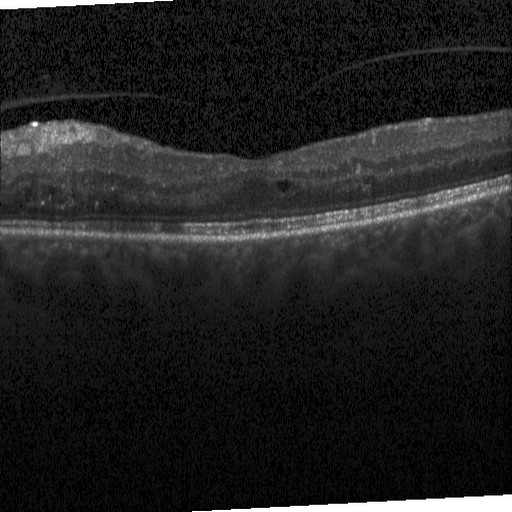 Centered on the fovea. Spectral-domain optical coherence tomography. Retinal OCT B-scan — Impression: diabetic macular edema (DME).